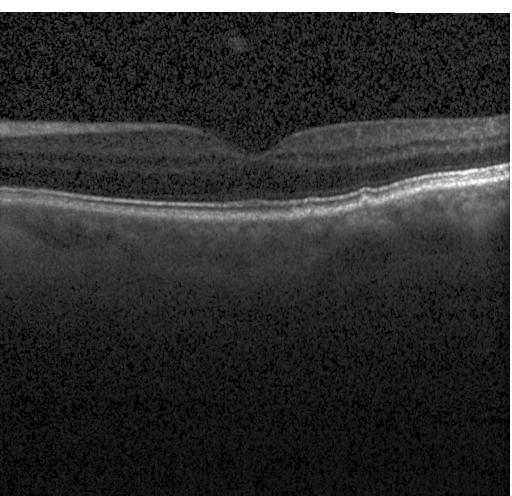 Spectral-domain OCT B-scan: drusen.